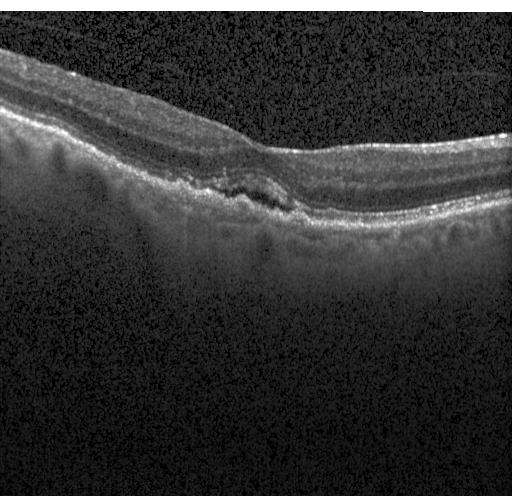

Acquired on a Heidelberg Spectralis. OCT B-scan. Horizontal scan through the fovea. Spectral-domain optical coherence tomography. Finding: a choroidal neovascular membrane.